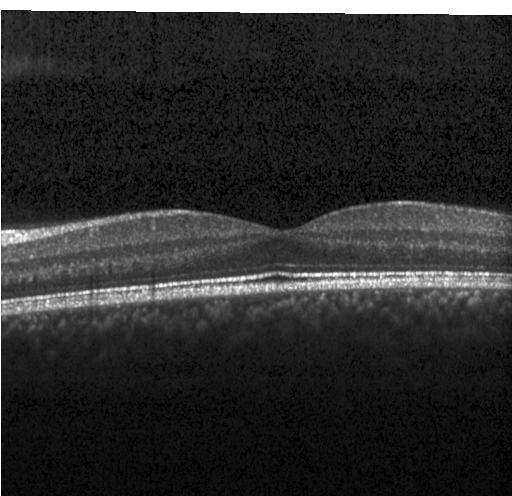
Spectral-domain optical coherence tomography; fovea-centered; optical coherence tomography B-scan; acquired on a Heidelberg Spectralis
Assessment: neither choroidal neovascularization, diabetic macular edema, nor drusen.